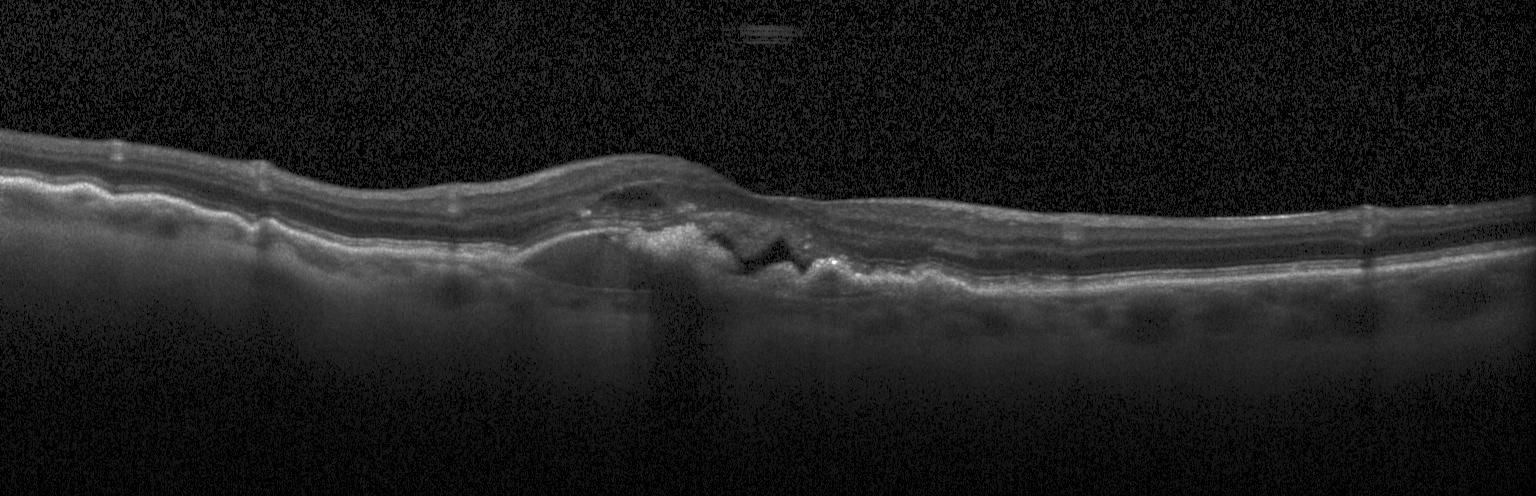
Spectral-domain OCT; retinal OCT B-scan; macular scan; acquired on a Heidelberg Spectralis. Assessment: a choroidal neovascular membrane.